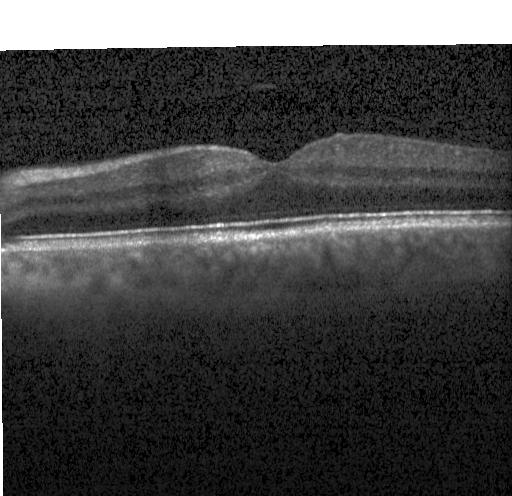
Diagnosis: no choroidal neovascularization, diabetic macular edema, or drusen.